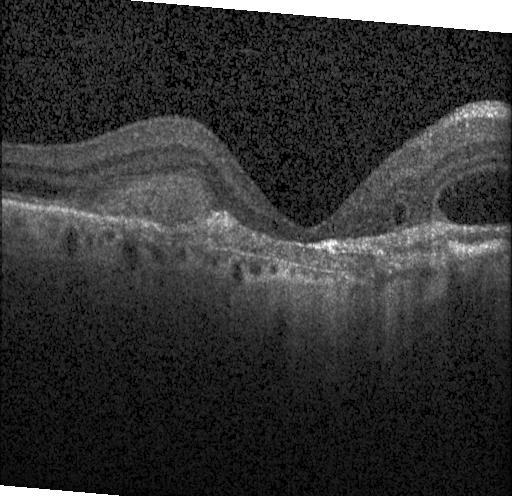

Macular OCT demonstrating choroidal neovascularization.